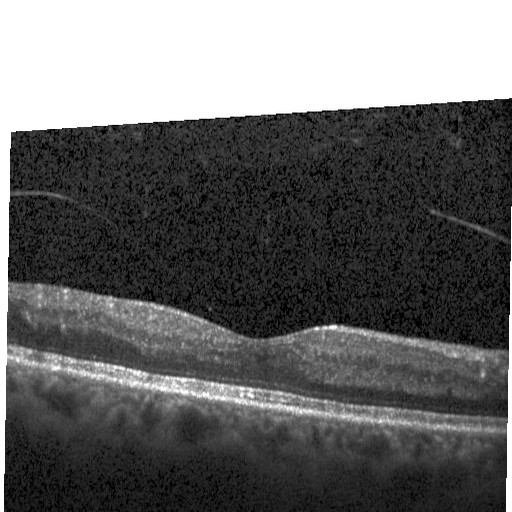 OCT B-scan. Finding: diabetic macular edema.